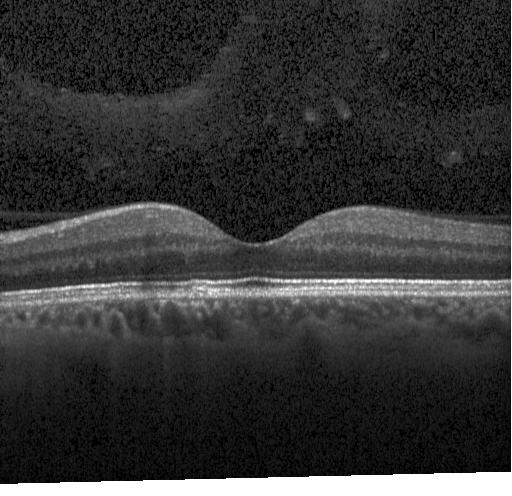

OCT line scan. Diagnosis: no choroidal neovascularization, diabetic macular edema, or drusen.